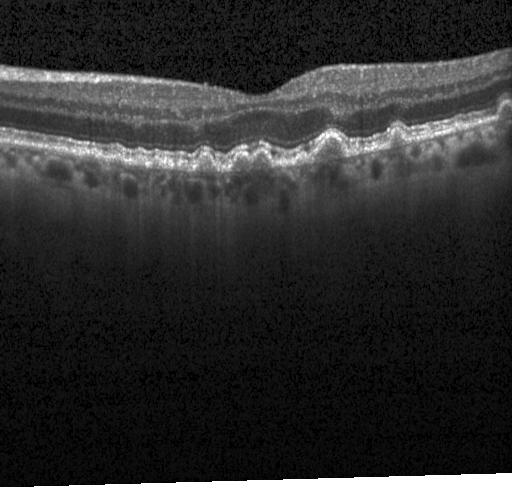
SD-OCT; OCT B-scan; horizontal scan through the fovea; acquired on a Heidelberg Spectralis — Sub-RPE drusenoid deposits.